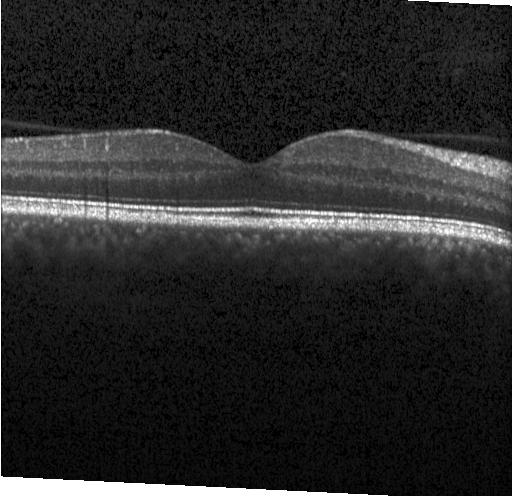

Retinal OCT cross-section.
Finding: neither choroidal neovascularization, diabetic macular edema, nor drusen.